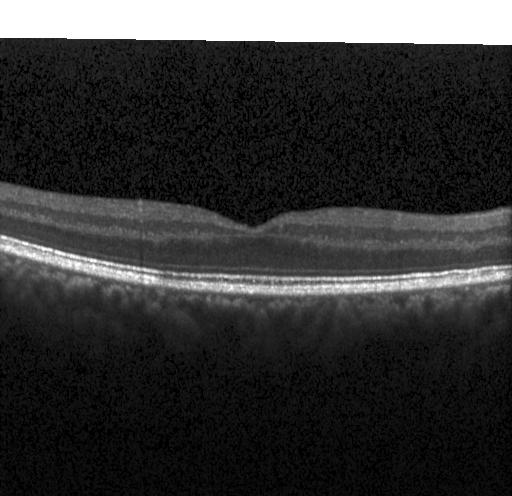
Horizontal scan through the fovea · SD-OCT · Heidelberg Spectralis · retinal OCT B-scan
This B-scan demonstrates no evidence of CNV, DME, or drusen.